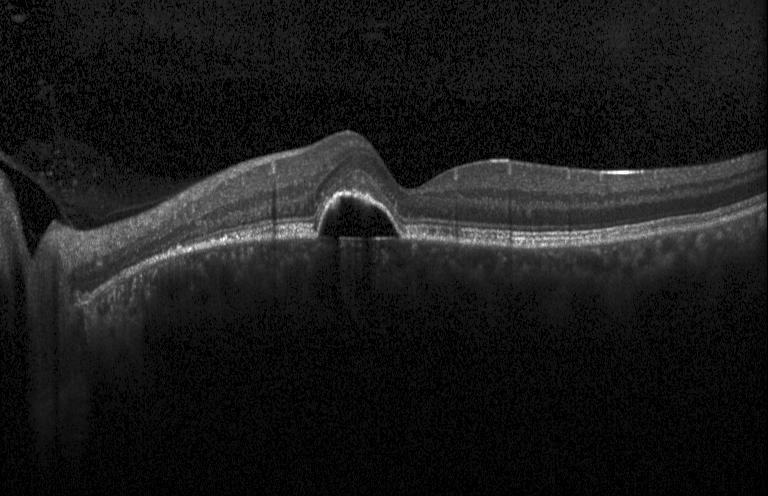 This B-scan demonstrates a choroidal neovascular membrane.